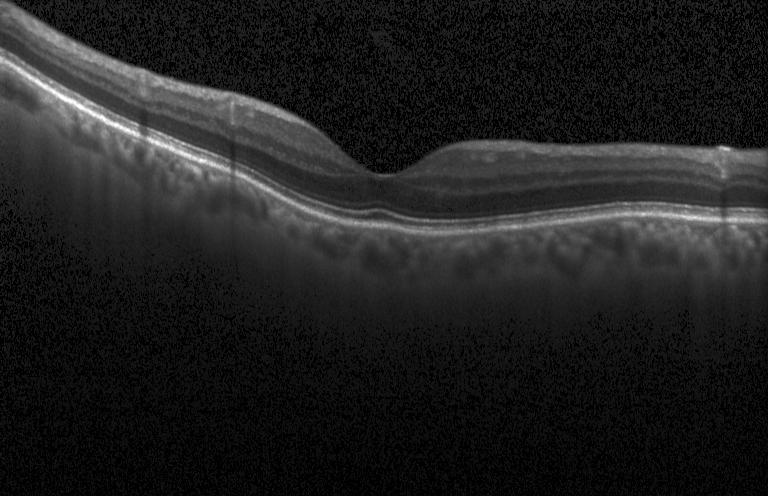

OCT B-scan. Acquired on a Heidelberg Spectralis. Spectral-domain optical coherence tomography
Macular OCT: no choroidal neovascularization, no diabetic macular edema, and no drusen.